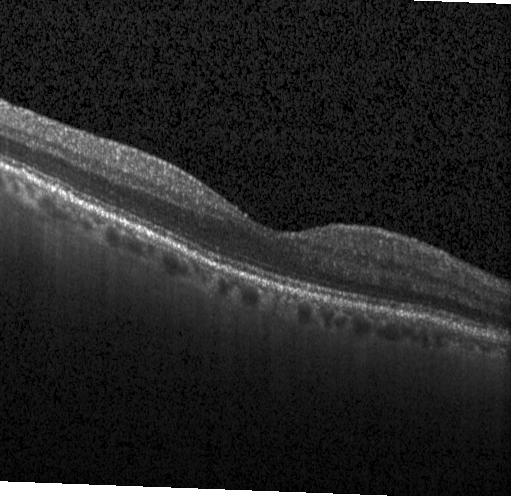 Retinal OCT cross-section, macular scan.
Impression: neither CNV, DME, nor drusen.